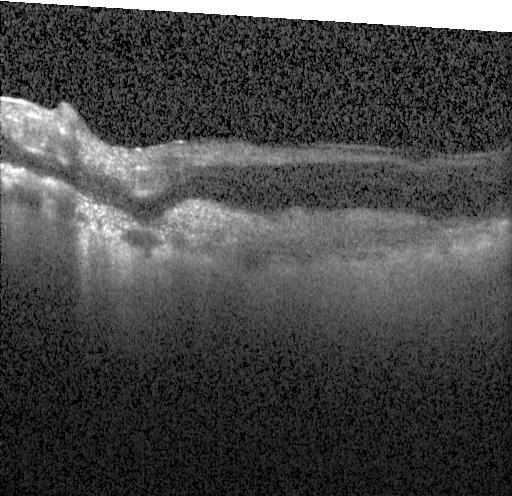

Optical coherence tomography scan
OCT finding: a choroidal neovascular membrane.